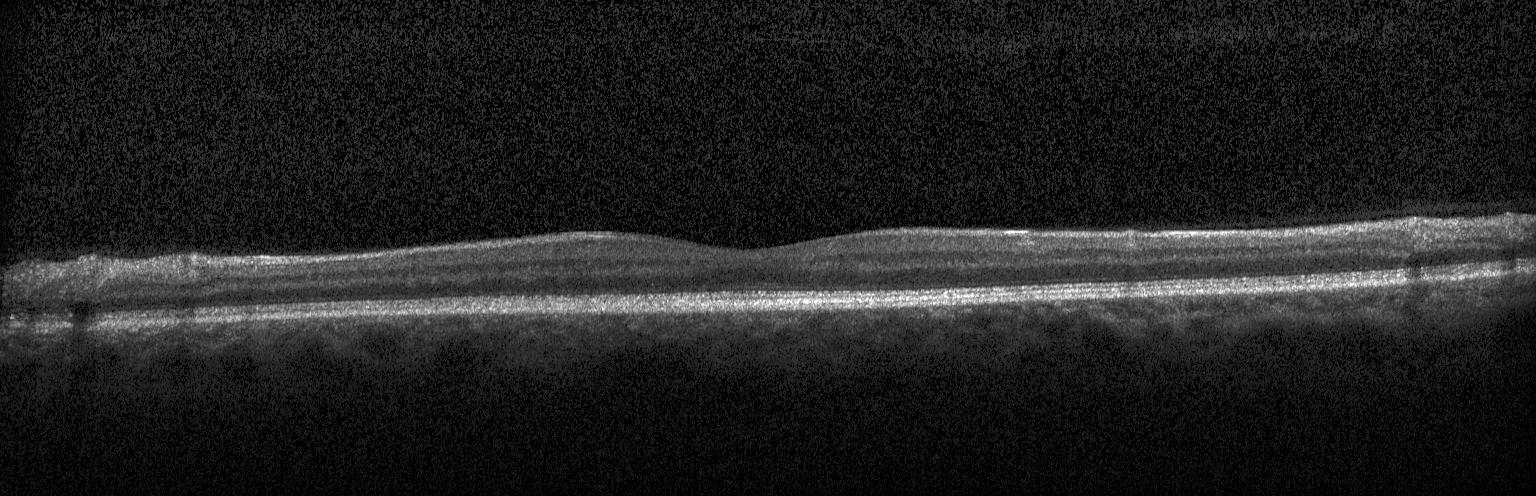 Optical coherence tomography B-scan
Dx: no CNV, no DME, and no drusen.